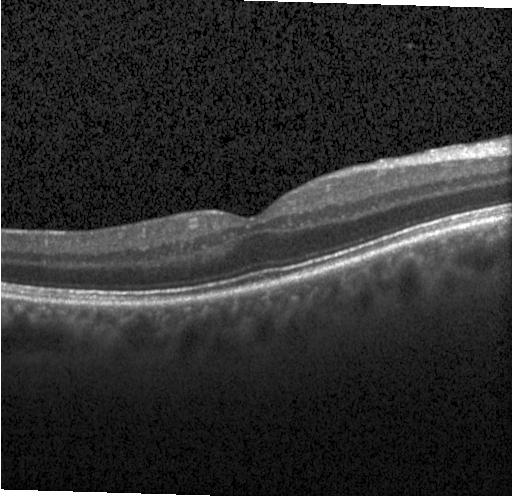
OCT line scan. Instrument: Heidelberg Spectralis. This B-scan demonstrates no choroidal neovascularization, diabetic macular edema, or drusen.